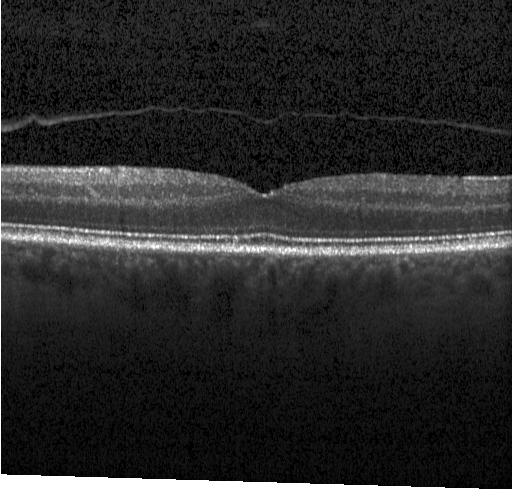
Spectral-domain OCT B-scan: neither choroidal neovascularization, diabetic macular edema, nor drusen.